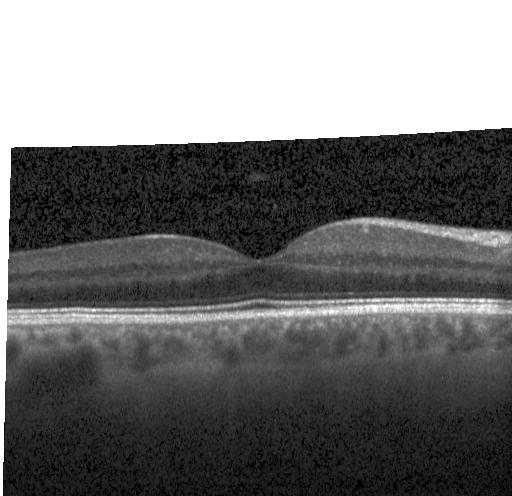

Heidelberg Spectralis OCT system. OCT B-scan. SD-OCT. Centered on the fovea — Impression: no choroidal neovascularization, no diabetic macular edema, and no drusen.